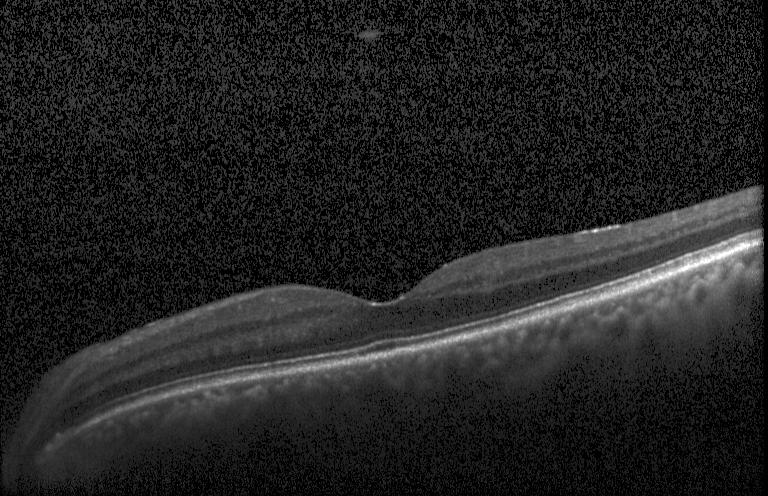
Macular OCT: no choroidal neovascularization, diabetic macular edema, or drusen.